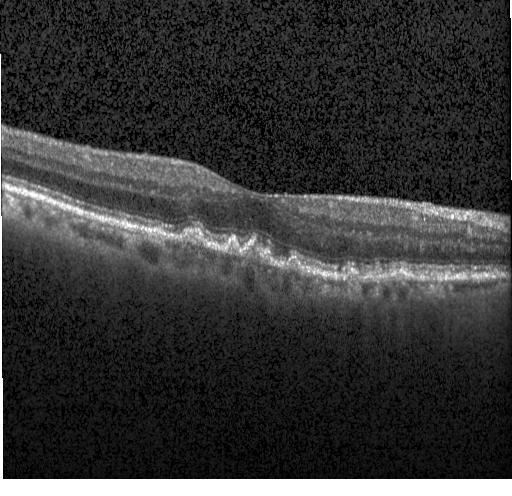

Spectral-domain optical coherence tomography. Optical coherence tomography B-scan. Through the macula — Assessment: multiple drusen.